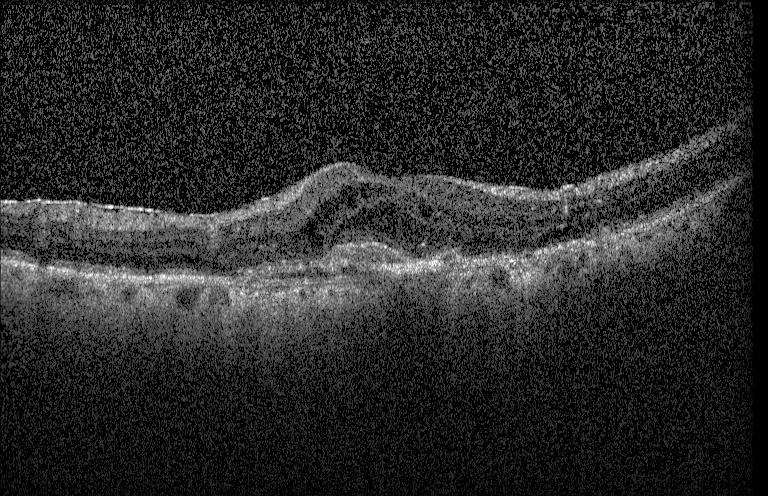 Horizontal scan through the fovea · optical coherence tomography scan — Diagnosis: a choroidal neovascular membrane.